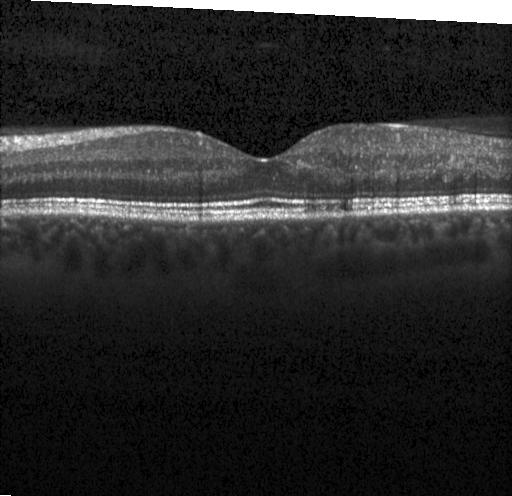 Optical coherence tomography scan; SD-OCT; Heidelberg Spectralis.
Assessment: neither CNV, DME, nor drusen.